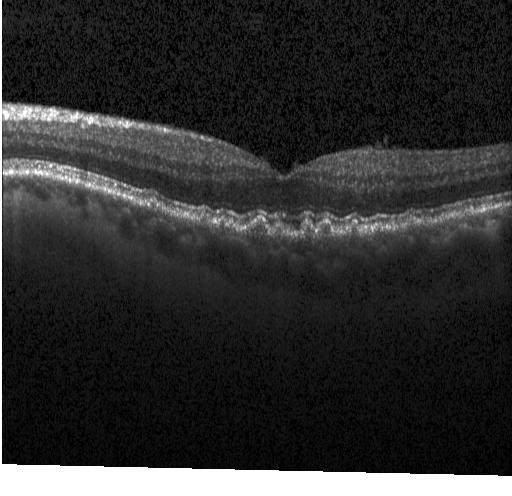

OCT line scan.
OCT finding: sub-RPE drusenoid deposits.